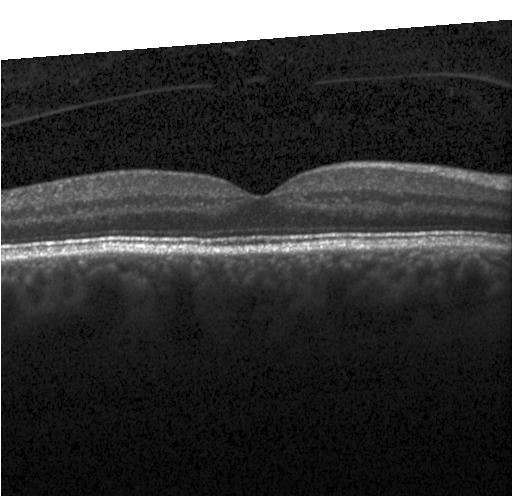

Dx: no evidence of choroidal neovascularization, diabetic macular edema, or drusen.